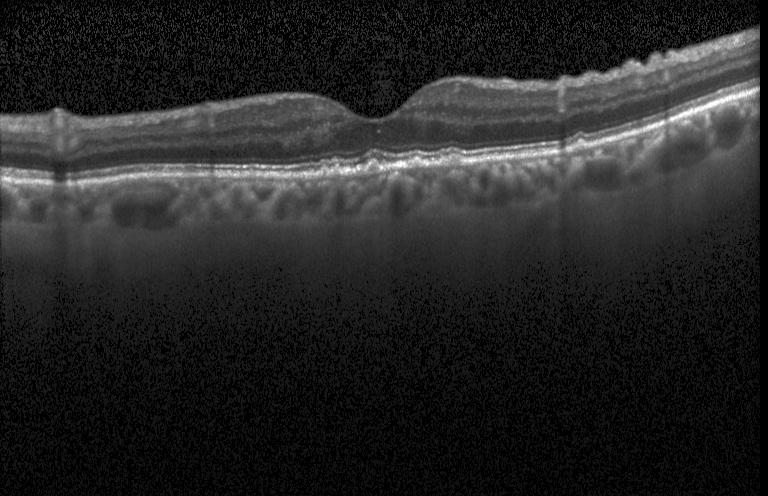
Impression: sub-RPE drusenoid deposits.